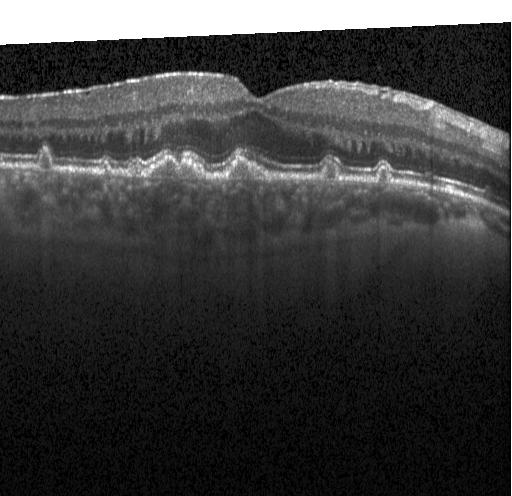
This B-scan demonstrates a choroidal neovascular membrane.